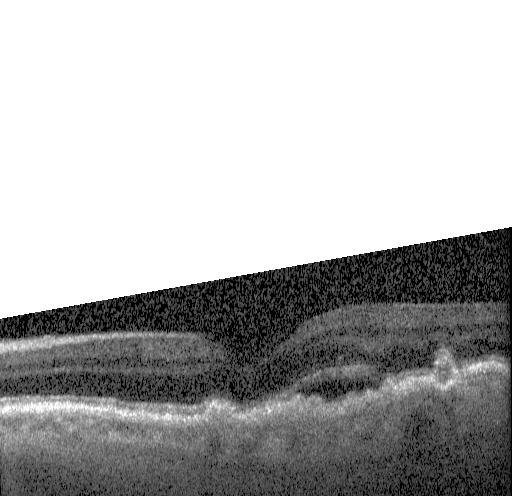

Diagnosis: choroidal neovascularization (CNV).